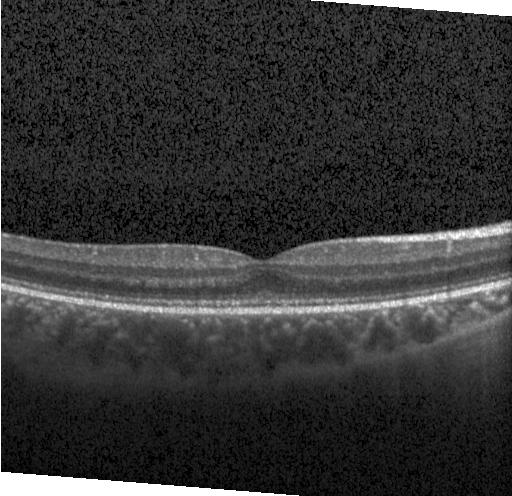
OCT B-scan — Assessment: no choroidal neovascularization, no diabetic macular edema, and no drusen.